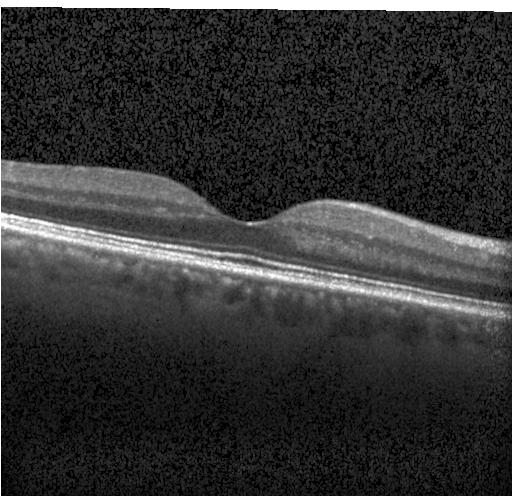

Optical coherence tomography scan.
Finding: no evidence of choroidal neovascularization, diabetic macular edema, or drusen.